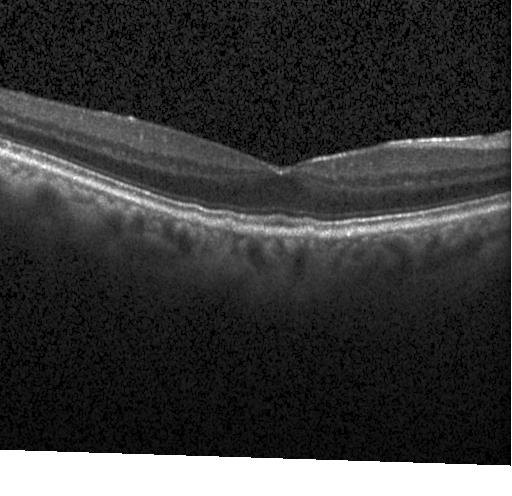

Fovea-centered; retinal OCT cross-section; SD-OCT
This B-scan demonstrates multiple drusen.